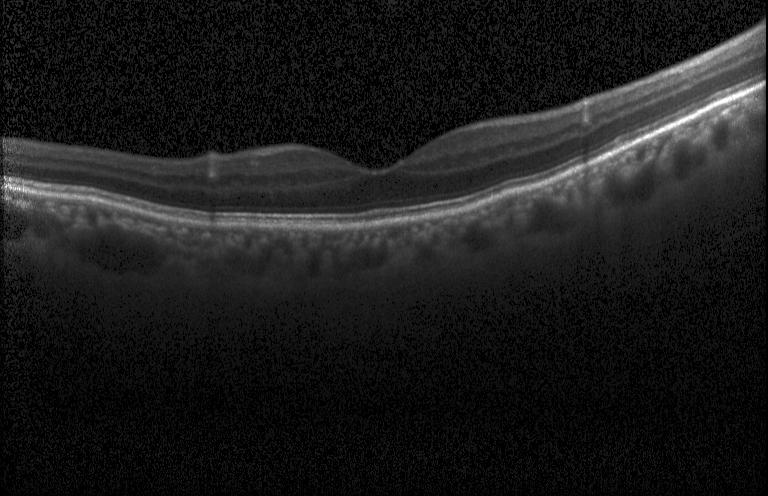

Retinal OCT B-scan
This B-scan demonstrates neither choroidal neovascularization, diabetic macular edema, nor drusen.